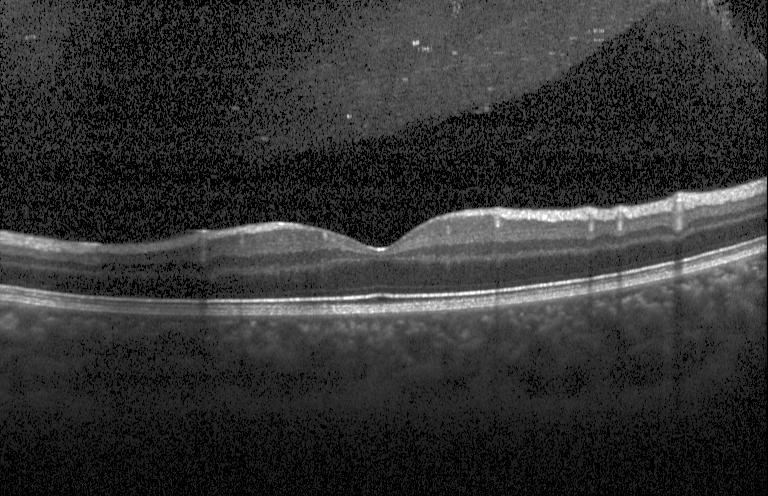 Retinal OCT B-scan.
Impression: no choroidal neovascularization, no diabetic macular edema, and no drusen.